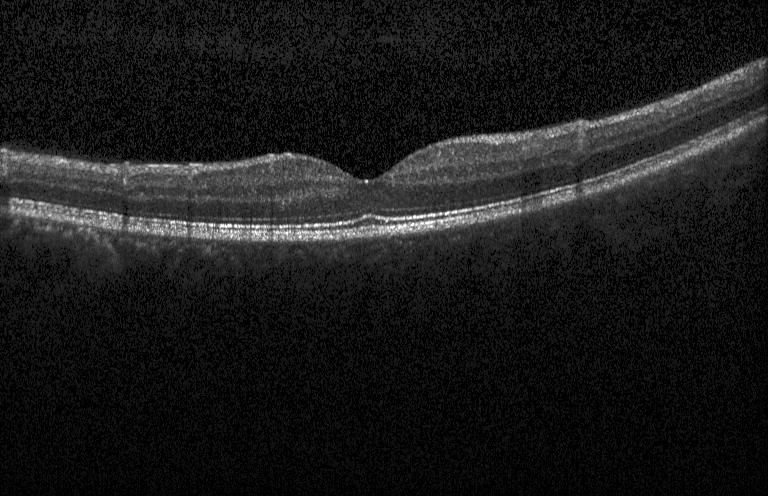

Fovea-centered, optical coherence tomography B-scan, spectral-domain optical coherence tomography, acquired on a Heidelberg Spectralis.
Diagnosis: no choroidal neovascularization, no diabetic macular edema, and no drusen.